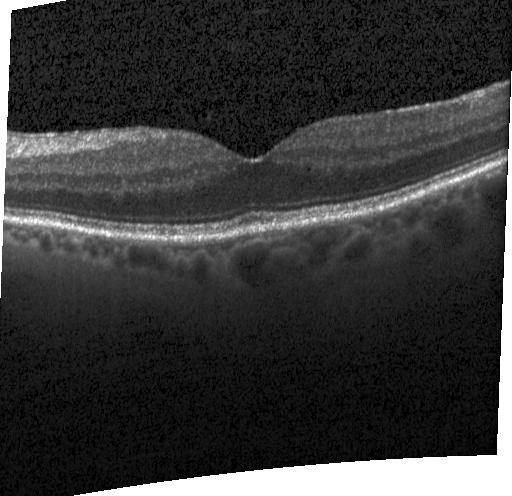 Diagnosis: no CNV, no DME, and no drusen.